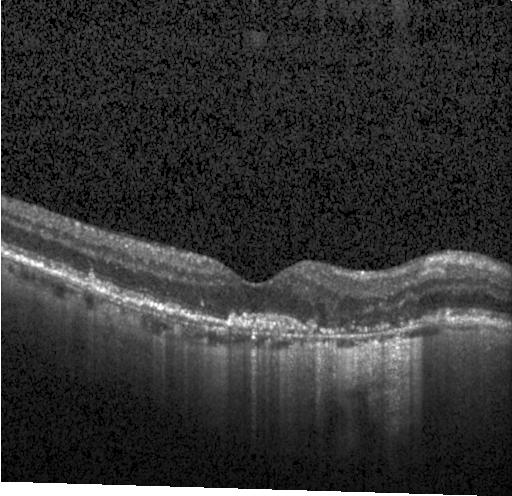

OCT B-scan — Diagnosis: a choroidal neovascular membrane.